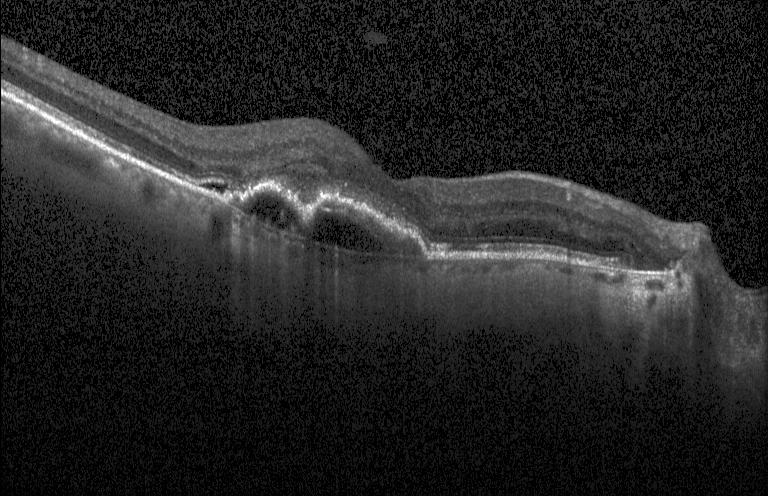

OCT line scan.
This B-scan demonstrates a choroidal neovascular membrane.